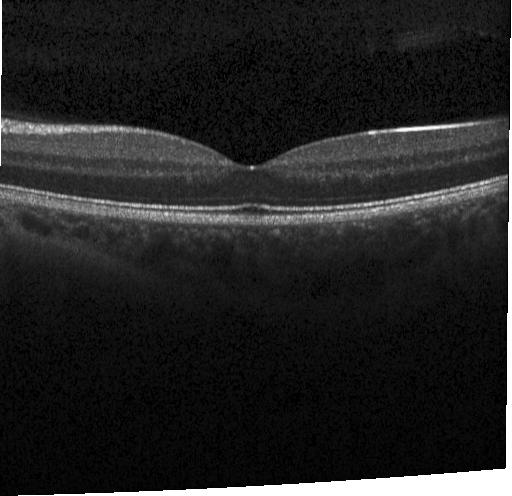
SD-OCT · fovea-centered · Heidelberg Spectralis · OCT B-scan — This B-scan demonstrates no evidence of choroidal neovascularization, diabetic macular edema, or drusen.